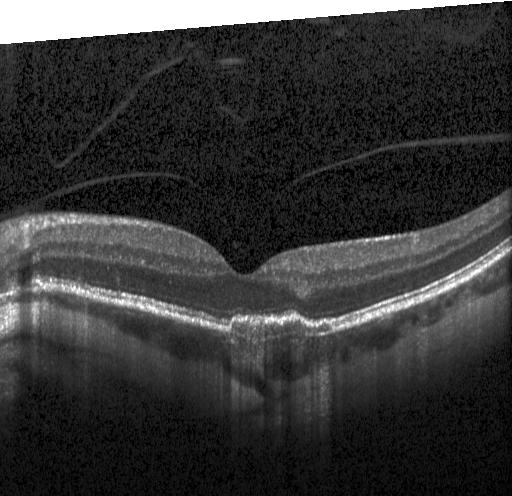

Assessment: CNV.